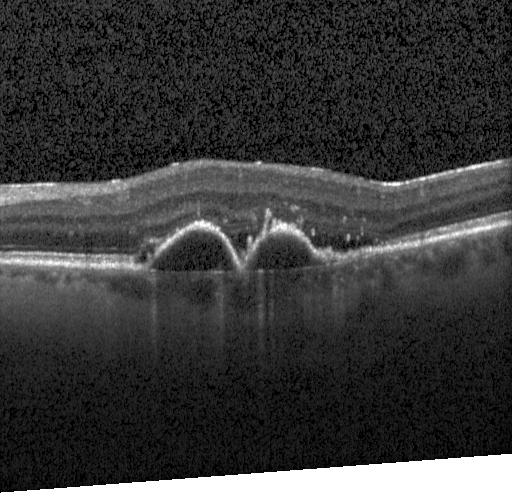 Macular scan, retinal OCT B-scan, spectral-domain OCT
Impression: a choroidal neovascular membrane.